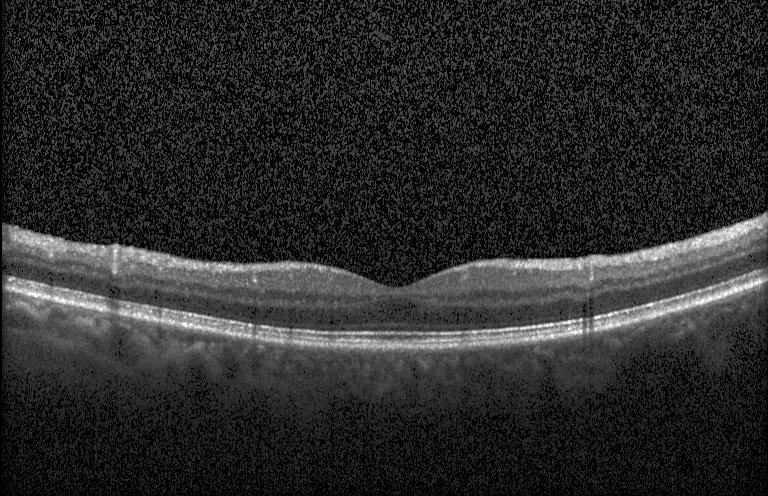

OCT line scan. Acquired on a Heidelberg Spectralis. Centered on the fovea
This B-scan demonstrates neither CNV, DME, nor drusen.